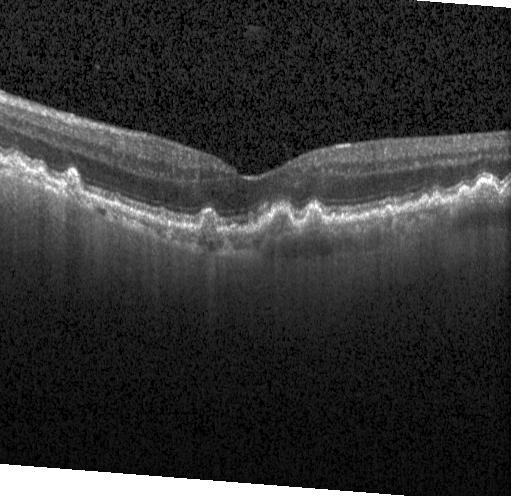
Retinal OCT cross-section · acquired on a Heidelberg Spectralis · SD-OCT — Diagnosis: multiple drusen.